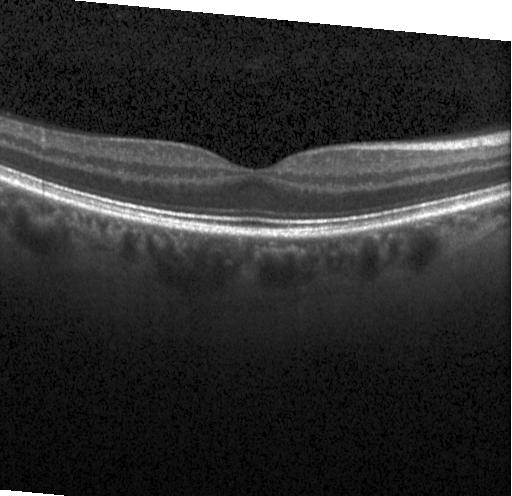 Horizontal scan through the fovea · OCT line scan · SD-OCT.
Assessment: no CNV, no DME, and no drusen.